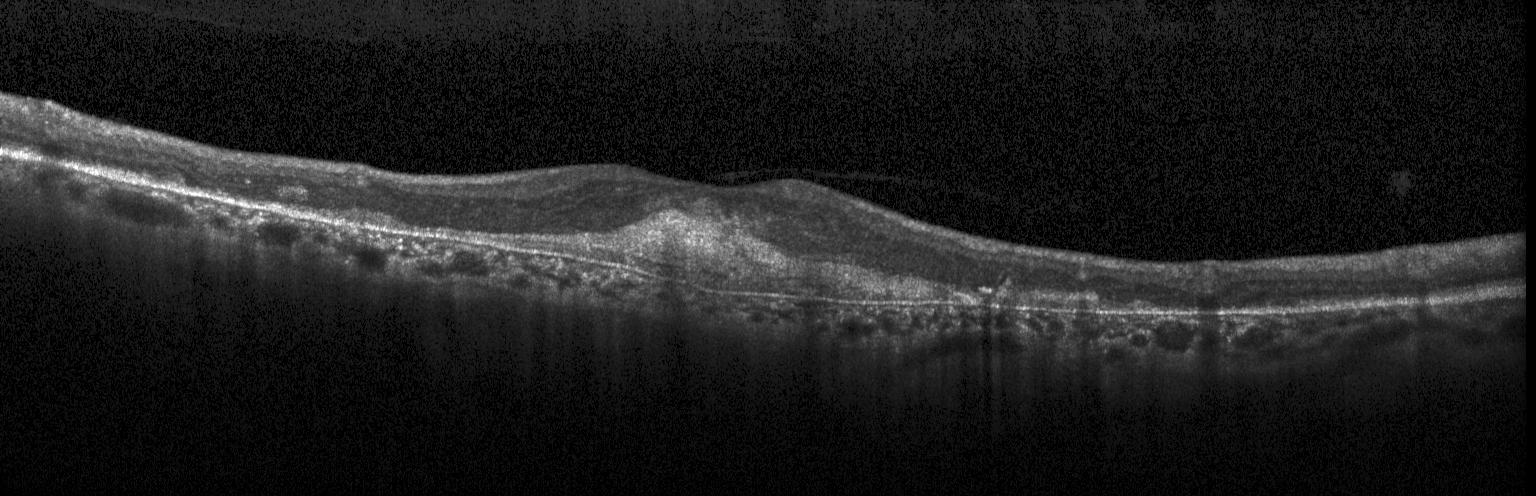 Macular OCT: a choroidal neovascular membrane.